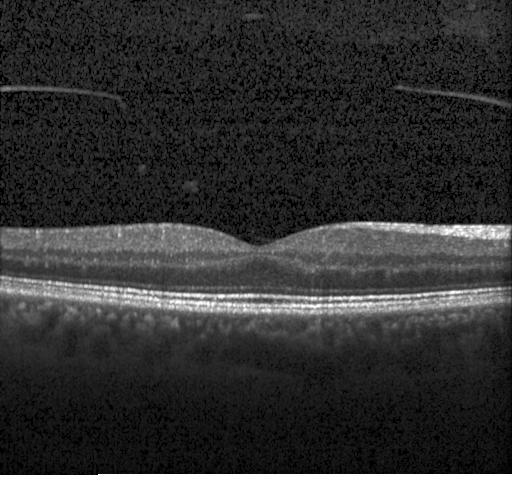 SD-OCT; OCT line scan; Heidelberg Spectralis OCT system; centered on the fovea
This B-scan demonstrates no choroidal neovascularization, no diabetic macular edema, and no drusen.